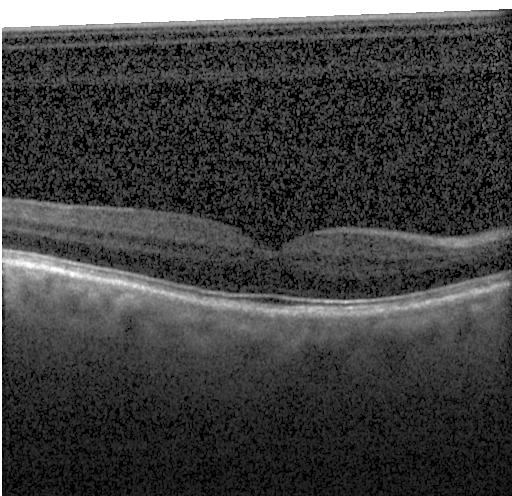 Centered on the fovea; OCT line scan; Heidelberg Spectralis.
Macular OCT: no evidence of CNV, DME, or drusen.